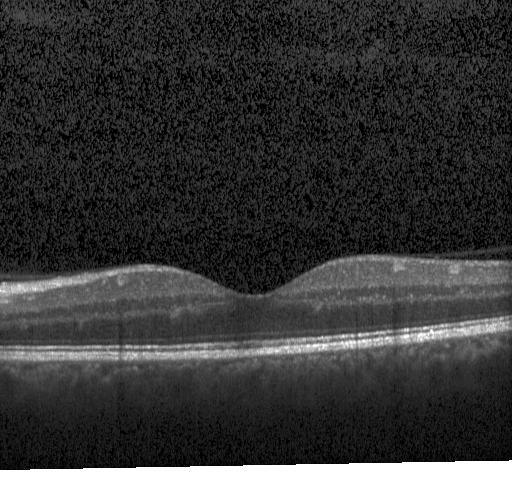
Neither CNV, DME, nor drusen.